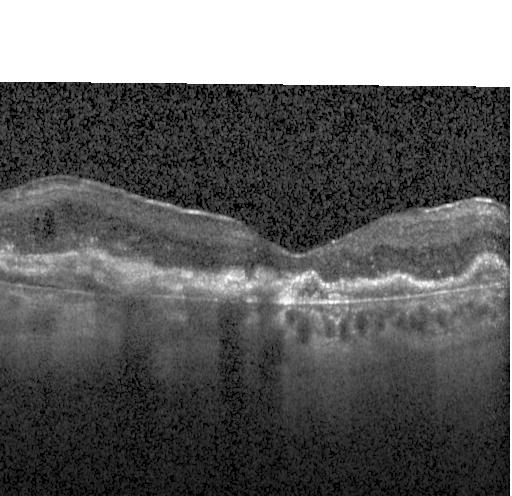
Retinal OCT cross-section showing choroidal neovascularization (CNV).